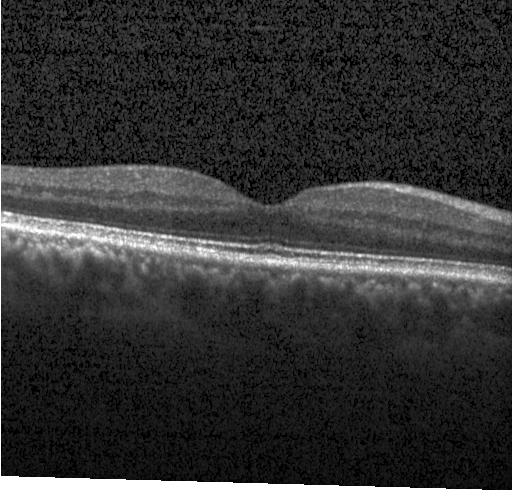 Optical coherence tomography B-scan. Macular scan
Impression: no choroidal neovascularization, no diabetic macular edema, and no drusen.